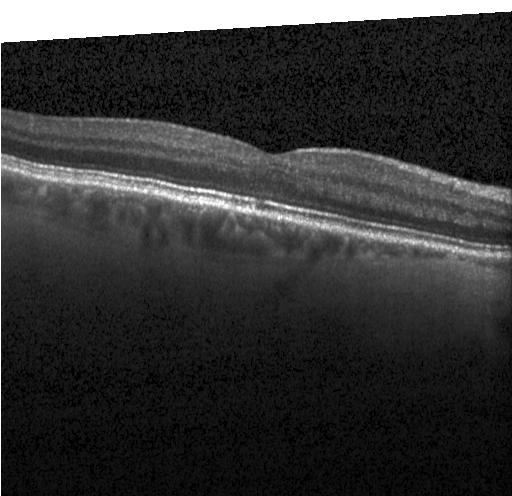 Retinal OCT B-scan.
Diagnosis: neither choroidal neovascularization, diabetic macular edema, nor drusen.